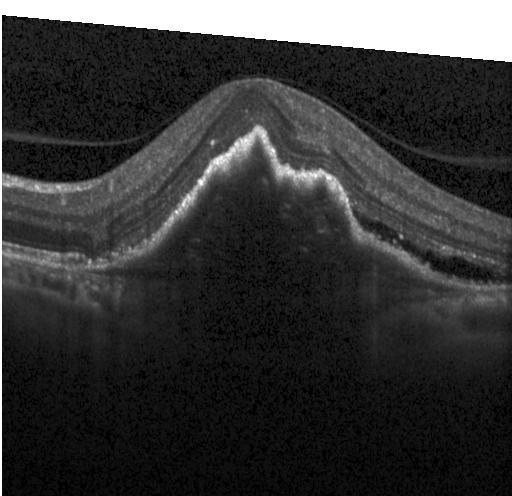 Macular OCT: CNV.